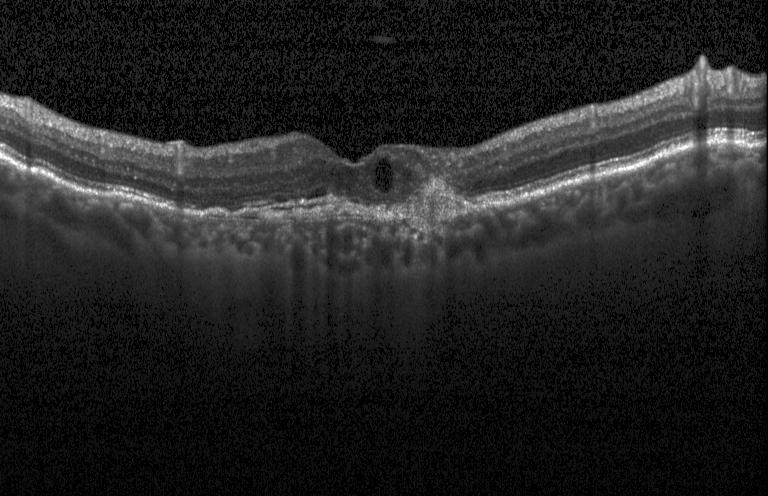
Heidelberg Spectralis OCT system; retinal OCT B-scan; spectral-domain optical coherence tomography
Diagnosis: choroidal neovascularization.